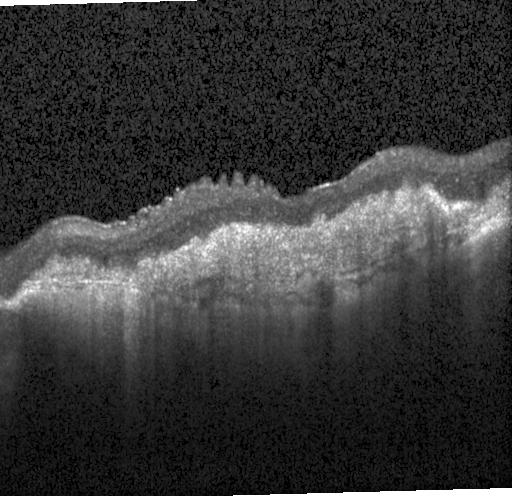
Through the macula · instrument: Heidelberg Spectralis · optical coherence tomography B-scan.
Finding: choroidal neovascularization.